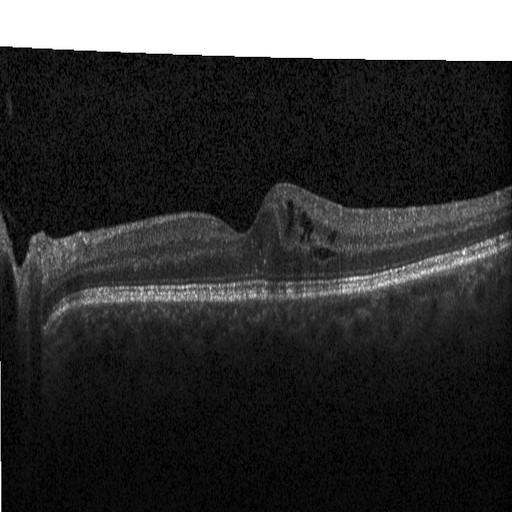
SD-OCT, optical coherence tomography scan — This B-scan demonstrates diabetic macular edema.